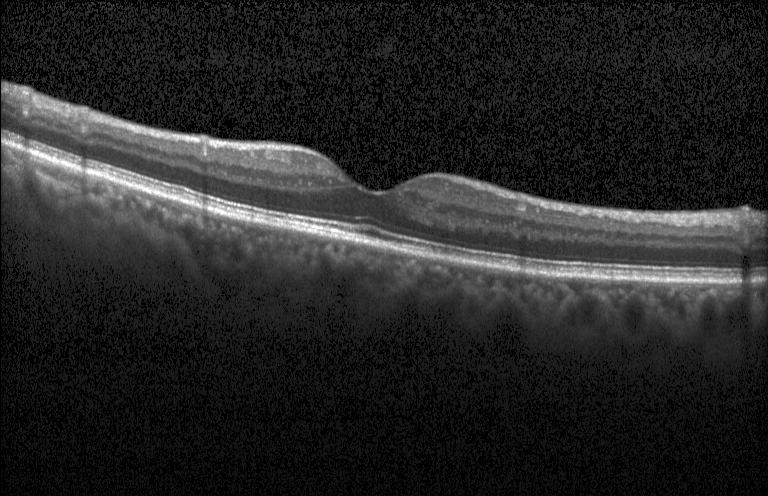 OCT B-scan; Heidelberg Spectralis; spectral-domain optical coherence tomography; horizontal scan through the fovea — Macular OCT: neither choroidal neovascularization, diabetic macular edema, nor drusen.